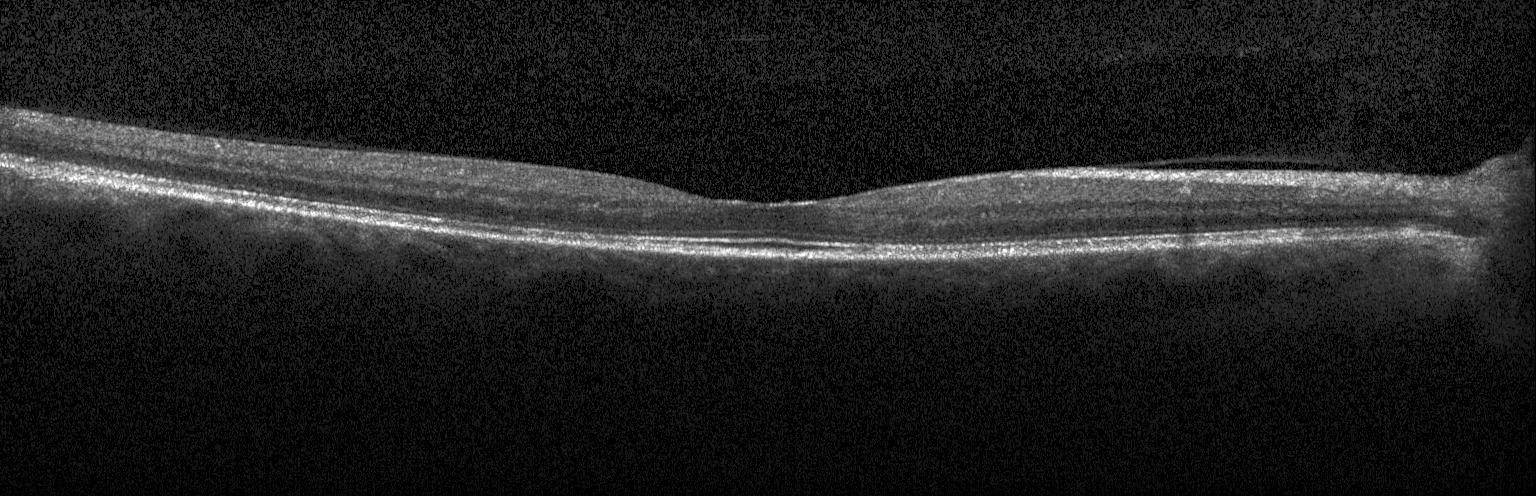

Impression: neither CNV, DME, nor drusen.